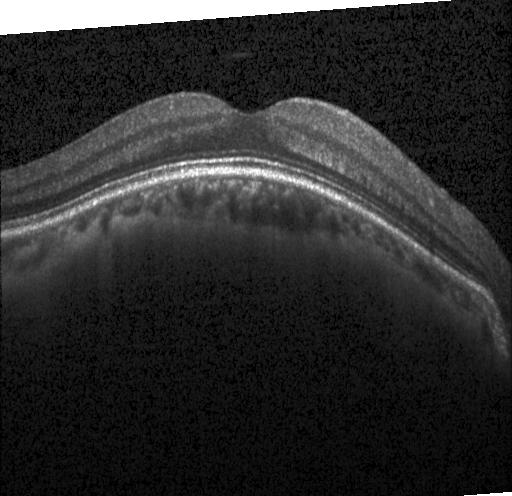
OCT finding: no choroidal neovascularization, no diabetic macular edema, and no drusen.